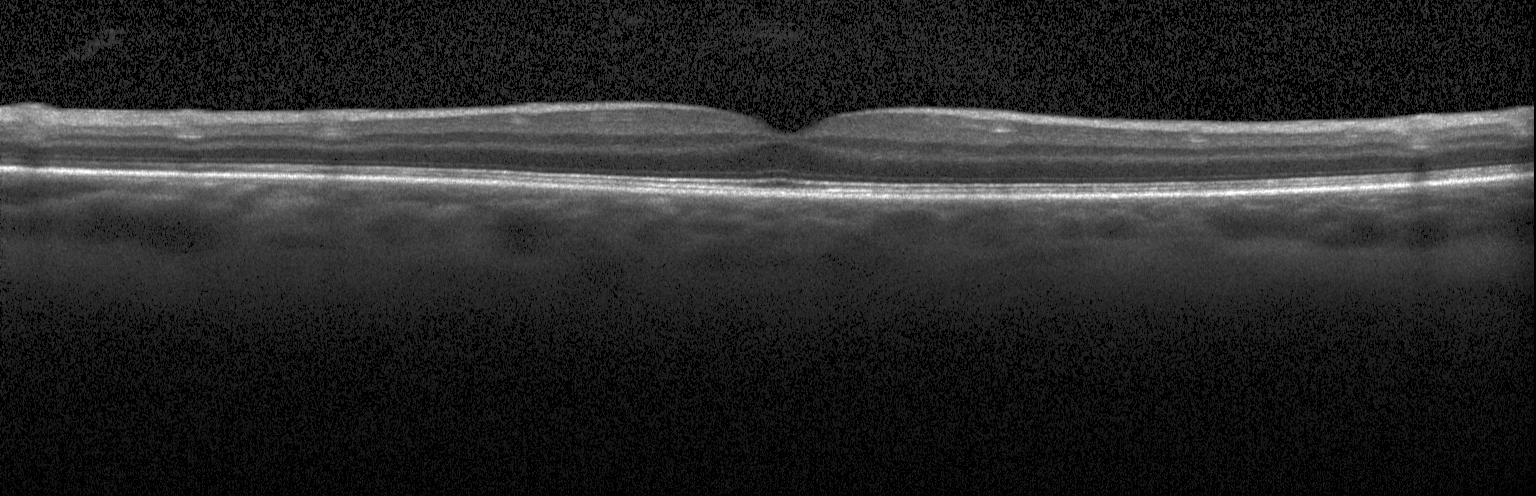

OCT B-scan · Heidelberg Spectralis OCT system · SD-OCT — This B-scan demonstrates neither choroidal neovascularization, diabetic macular edema, nor drusen.